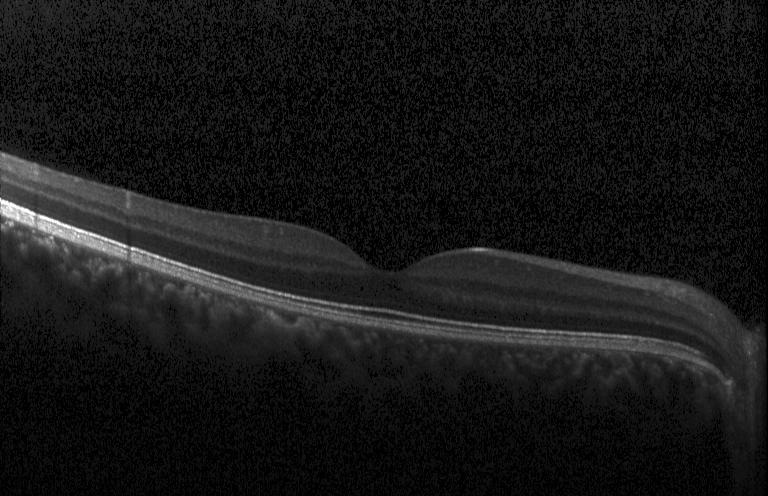

Optical coherence tomography B-scan. Spectral-domain OCT. Fovea-centered
Diagnosis: no choroidal neovascularization, diabetic macular edema, or drusen.